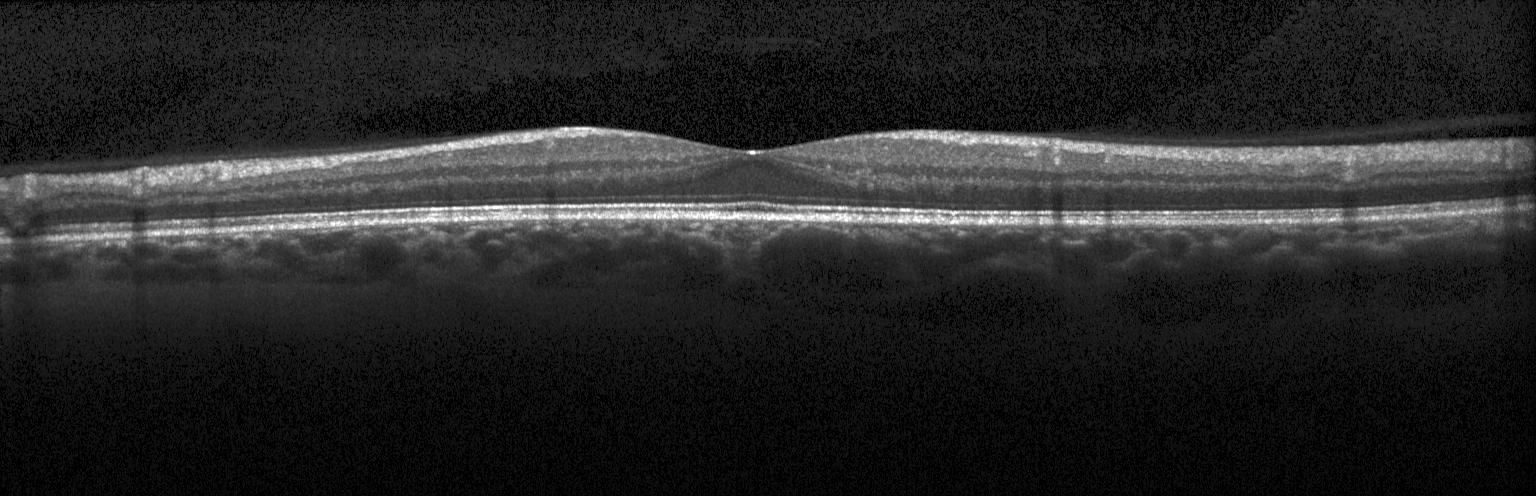 This B-scan demonstrates no choroidal neovascularization, diabetic macular edema, or drusen.